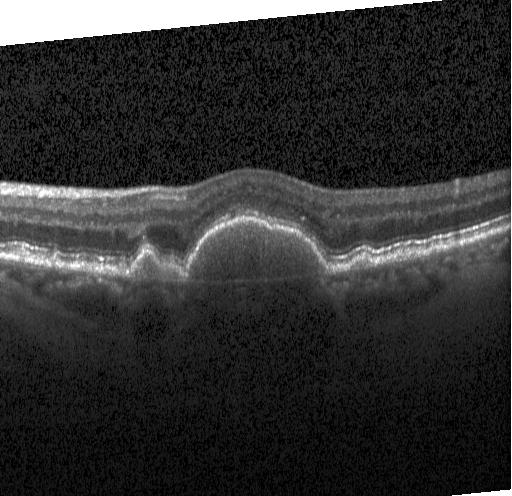
SD-OCT · fovea-centered · OCT line scan.
Diagnosis: a choroidal neovascular membrane.